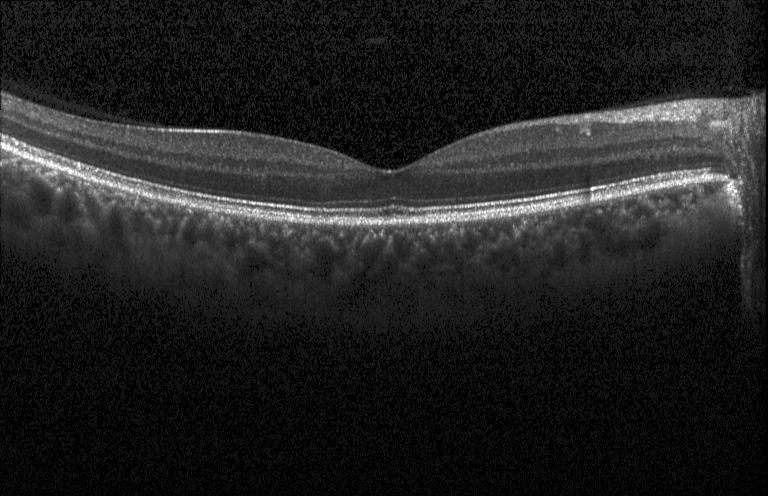
Heidelberg Spectralis. Retinal OCT B-scan — Assessment: neither choroidal neovascularization, diabetic macular edema, nor drusen.